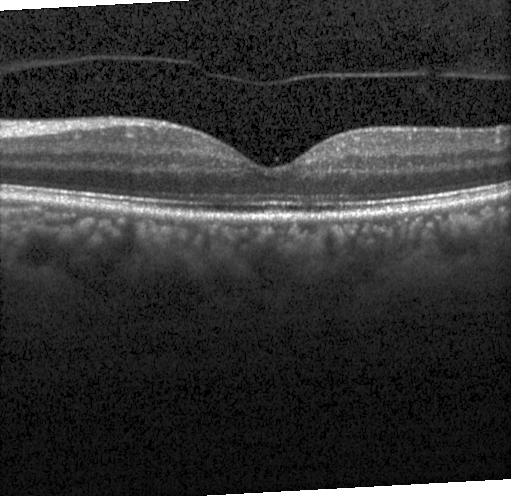

Spectral-domain OCT B-scan: no evidence of CNV, DME, or drusen.